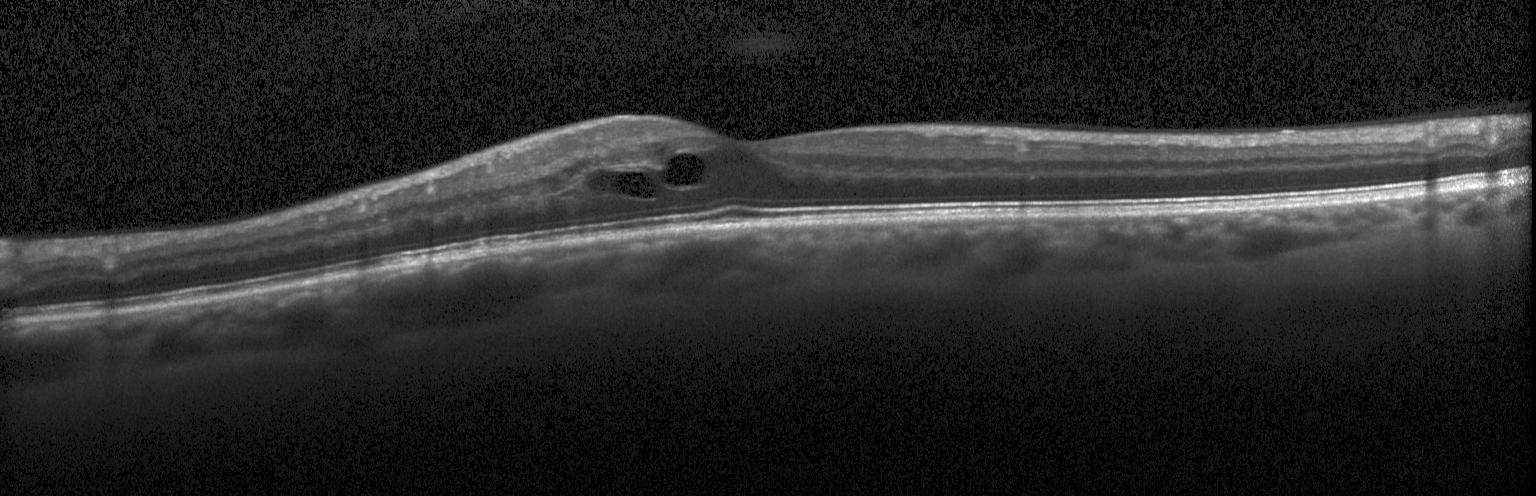

OCT finding: diabetic macular edema (DME).